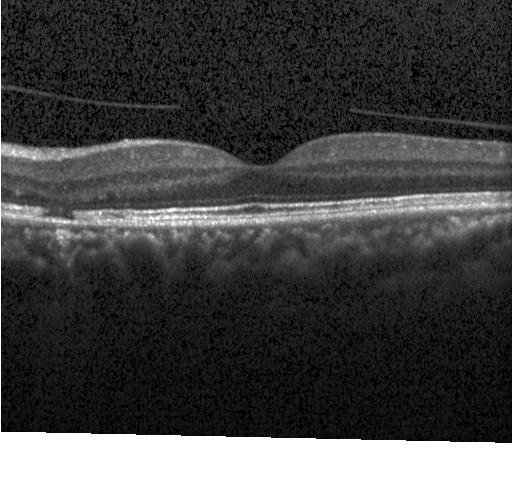
Retinal OCT cross-section
Impression: neither CNV, DME, nor drusen.